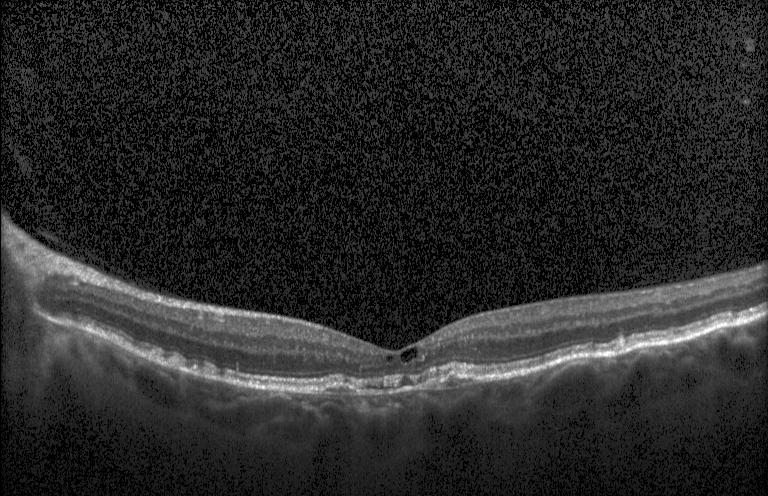

OCT B-scan showing a choroidal neovascular membrane.